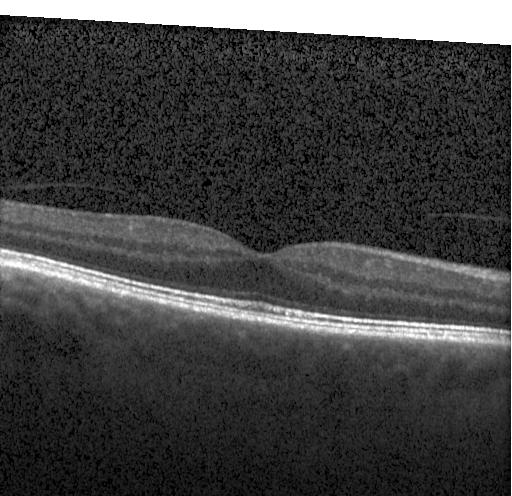

Spectral-domain OCT. Retinal OCT B-scan. Heidelberg Spectralis OCT system
Finding: no choroidal neovascularization, diabetic macular edema, or drusen.